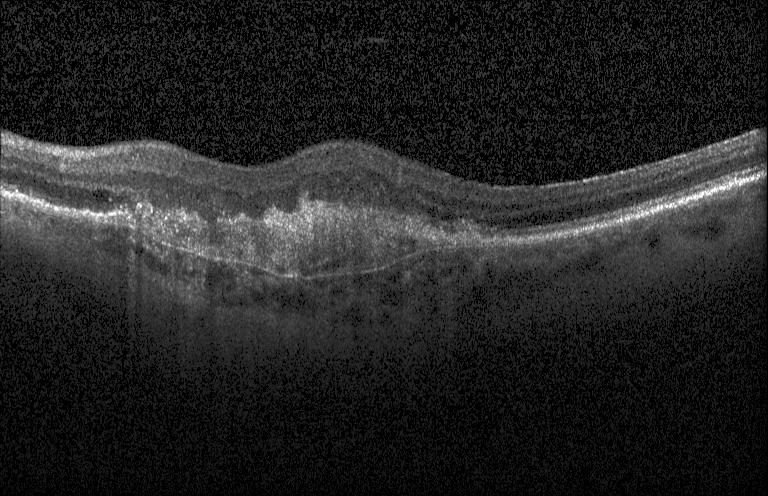
Optical coherence tomography B-scan
This B-scan demonstrates a choroidal neovascular membrane.